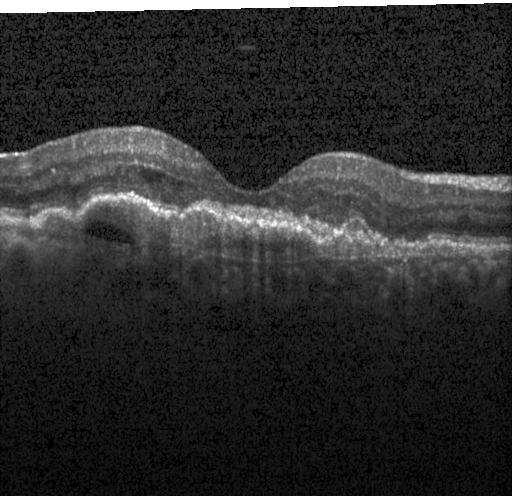
Retinal OCT B-scan
Dx: a choroidal neovascular membrane.